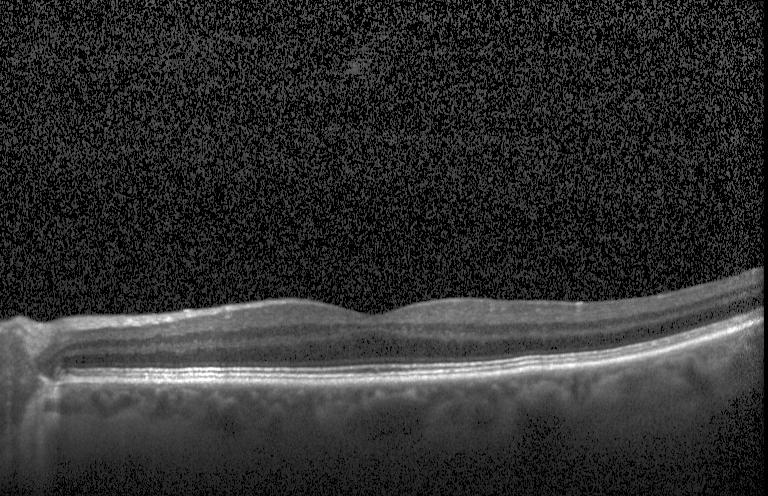 Heidelberg Spectralis OCT system; optical coherence tomography B-scan.
Assessment: no CNV, no DME, and no drusen.